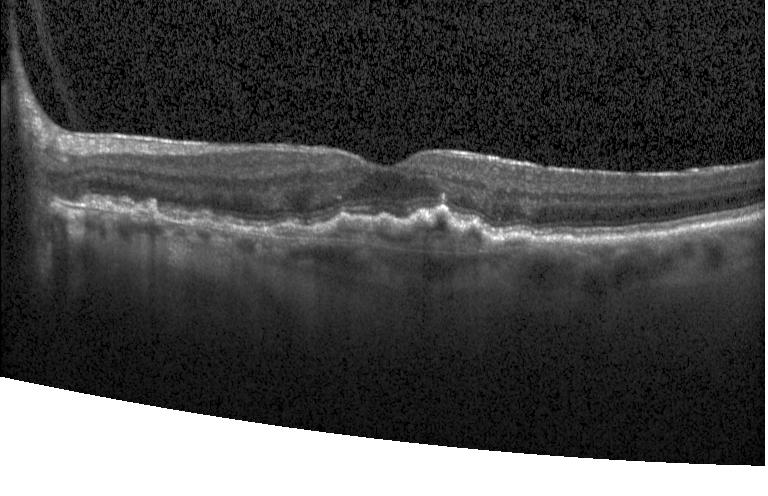
OCT scan showing choroidal neovascularization.